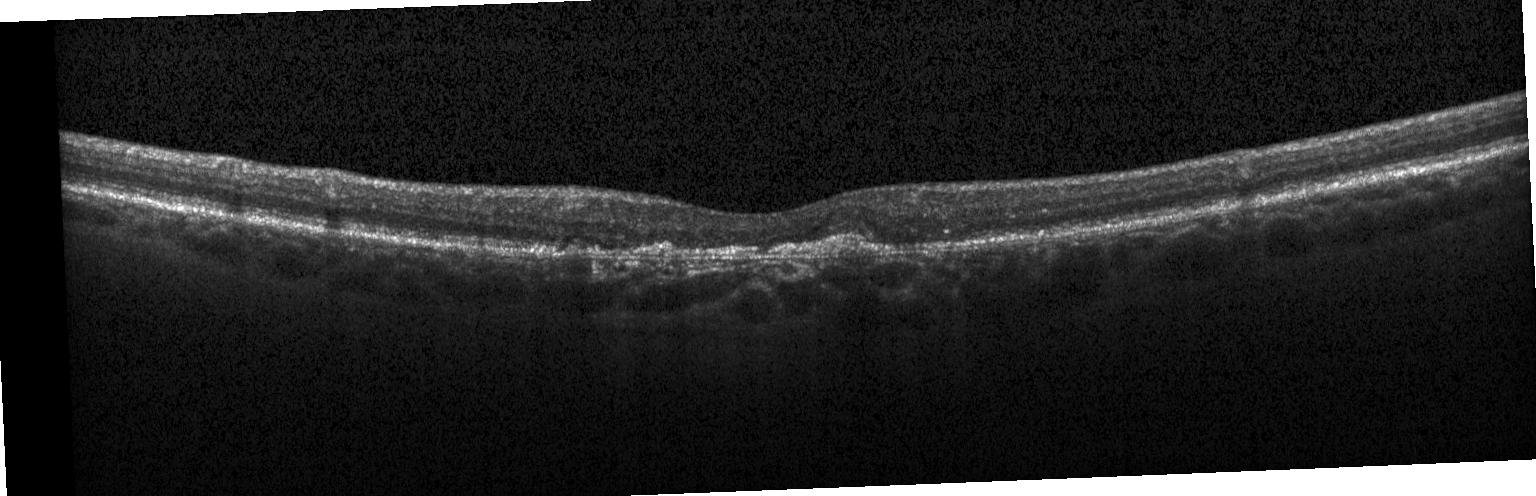

Retinal OCT cross-section. Acquired on a Heidelberg Spectralis — OCT finding: choroidal neovascularization.